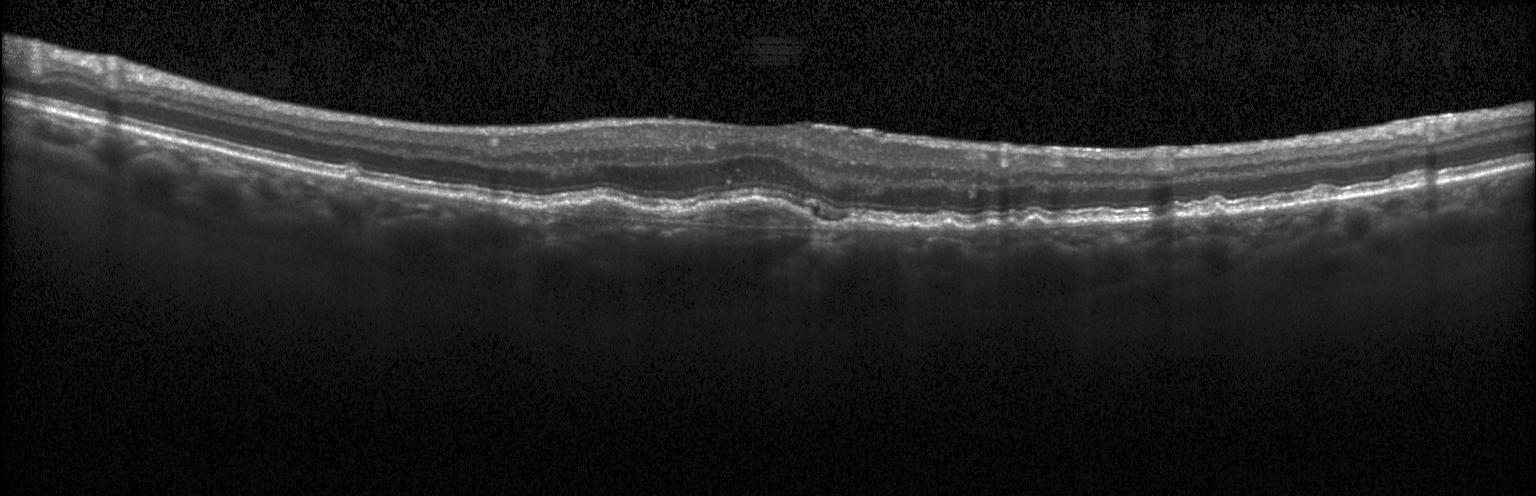 Retinal OCT B-scan. Spectral-domain OCT.
The scan shows choroidal neovascularization.